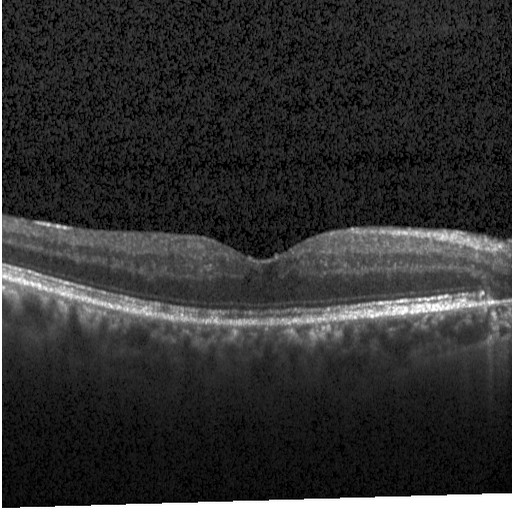

Acquired on a Heidelberg Spectralis, optical coherence tomography scan
Assessment: diabetic macular edema.